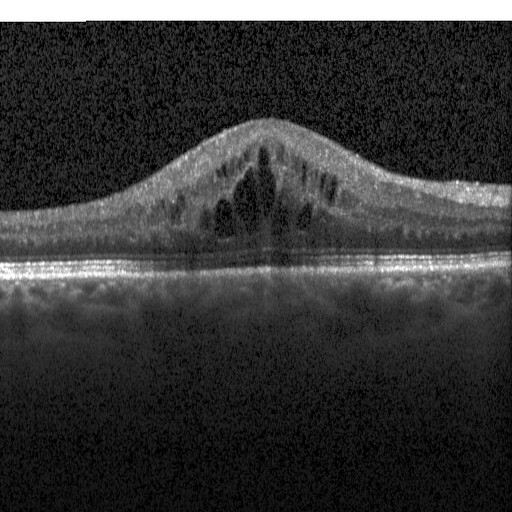
Optical coherence tomography scan
Finding: diabetic macular edema.